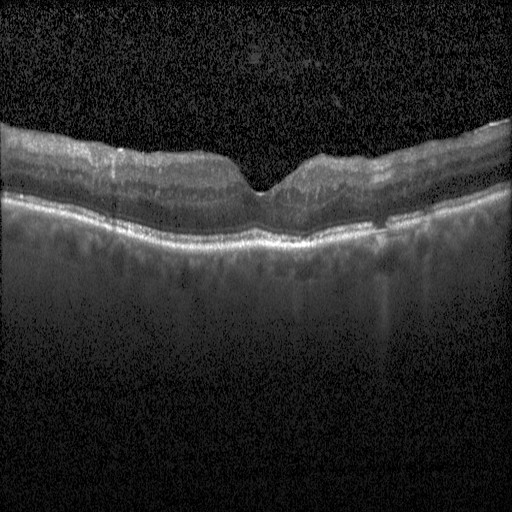

Optical coherence tomography scan. Spectral-domain OCT. Diabetic macular edema.